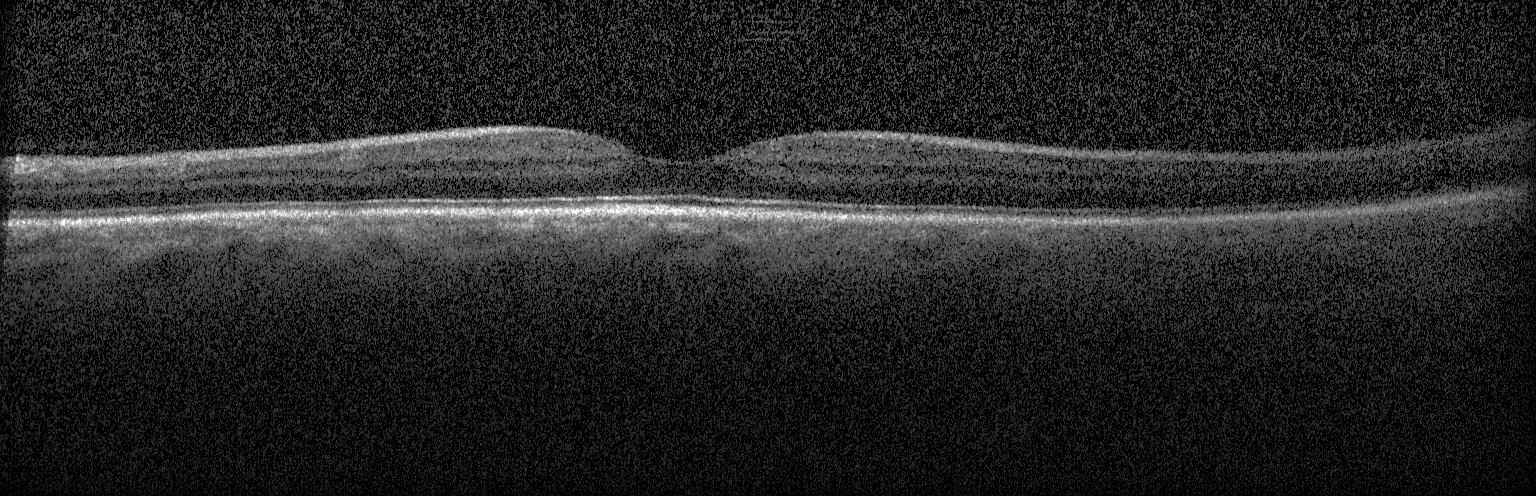
Finding: no evidence of CNV, DME, or drusen.